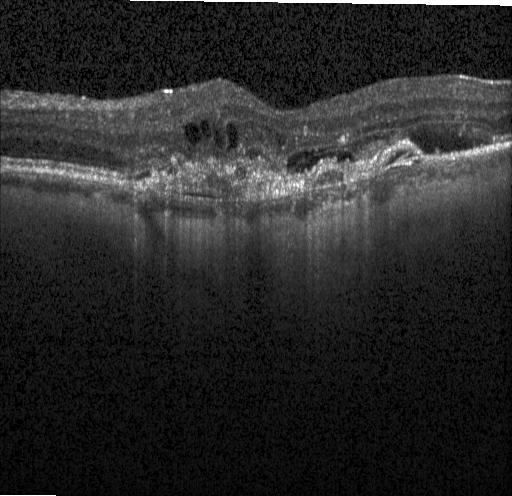
This B-scan demonstrates a choroidal neovascular membrane.